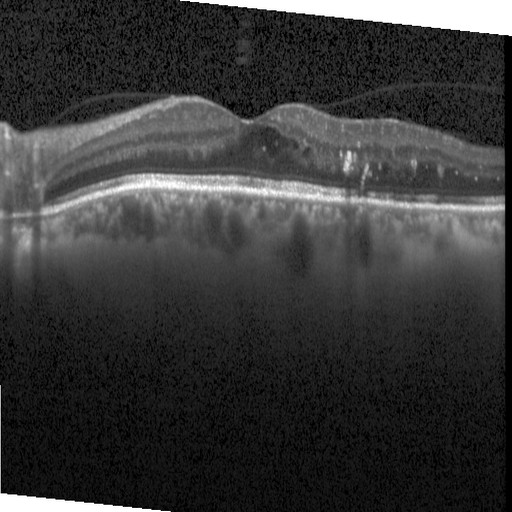
Finding: diabetic macular edema (DME).